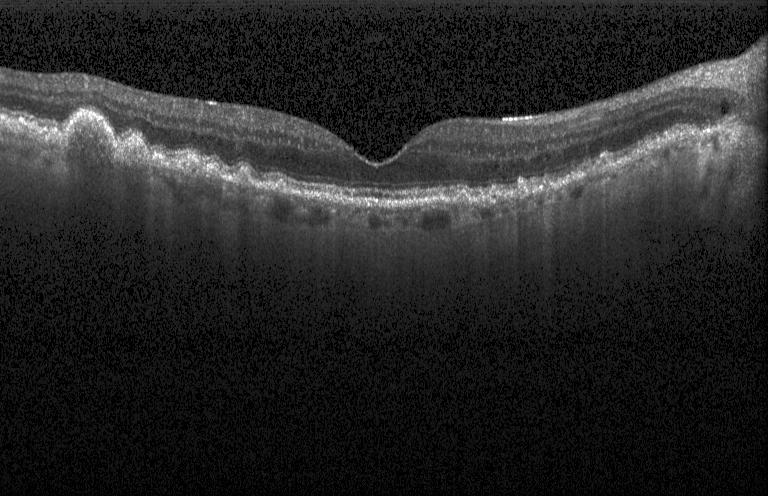 Through the macula; spectral-domain OCT; retinal OCT cross-section. Multiple drusen.